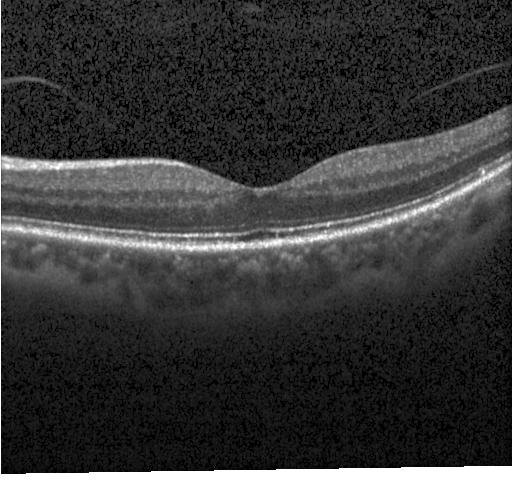

Finding: no choroidal neovascularization, no diabetic macular edema, and no drusen.